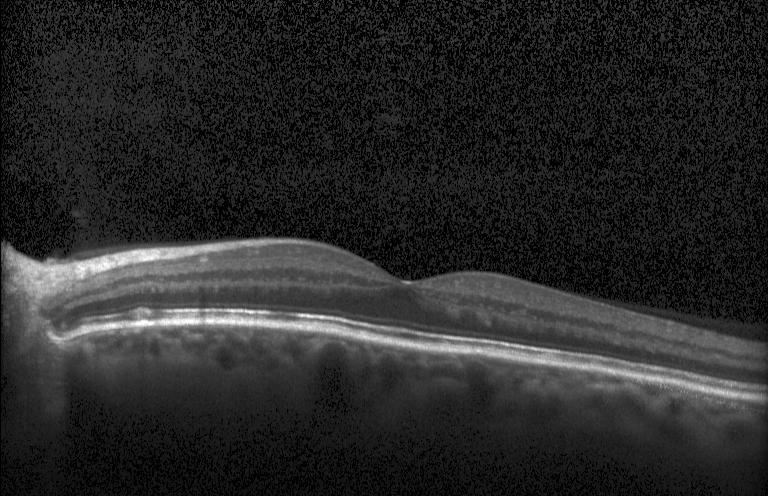
Retinal OCT cross-section showing no choroidal neovascularization, diabetic macular edema, or drusen.